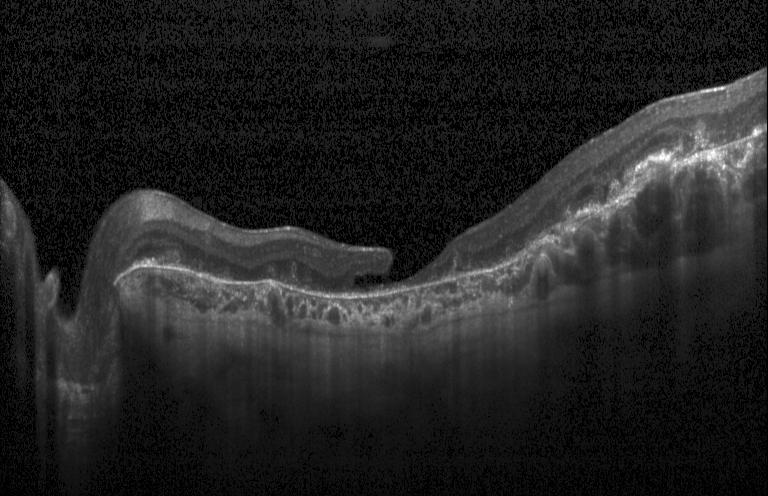

Spectral-domain OCT; retinal OCT B-scan; horizontal scan through the fovea; acquired on a Heidelberg Spectralis. Finding: choroidal neovascularization.